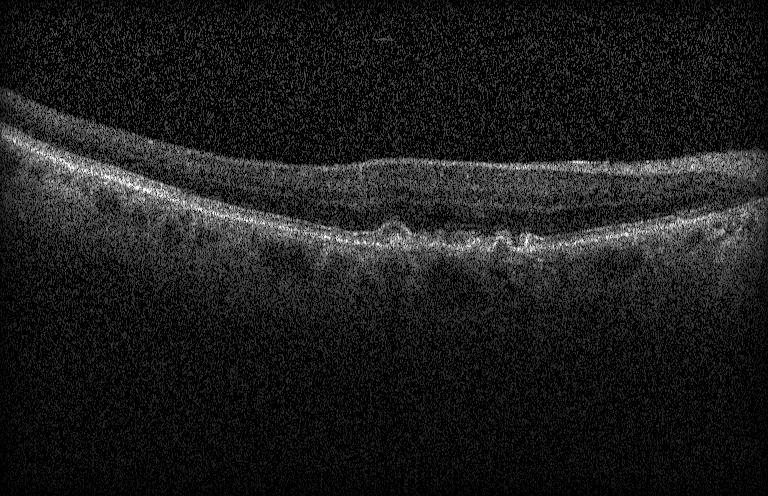

Impression: multiple drusen.